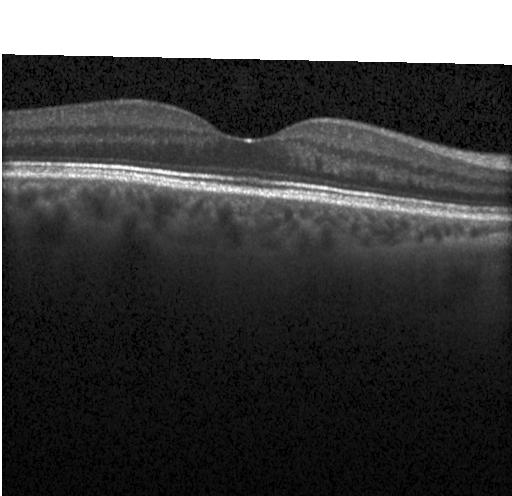 Retinal OCT B-scan.
Macular OCT: no choroidal neovascularization, no diabetic macular edema, and no drusen.